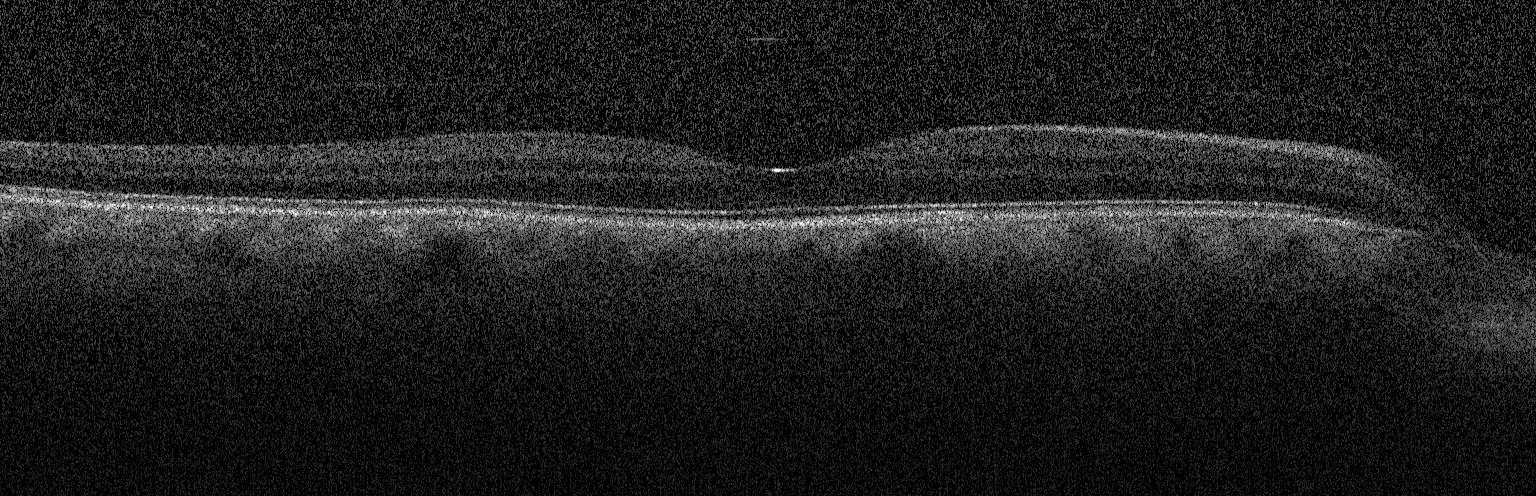

Assessment: no CNV, DME, or drusen.